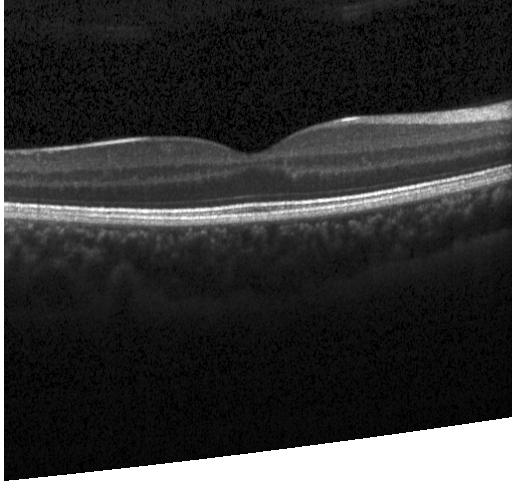

OCT line scan, spectral-domain optical coherence tomography — No CNV, DME, or drusen.